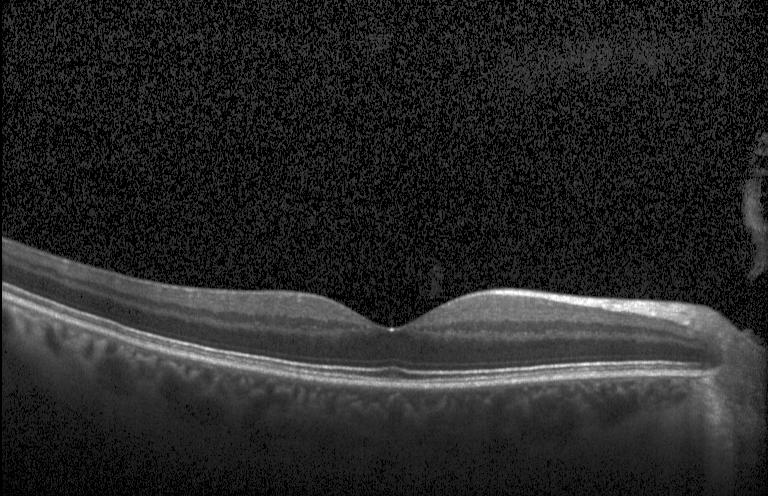

Optical coherence tomography B-scan · fovea-centered. Impression: neither CNV, DME, nor drusen.